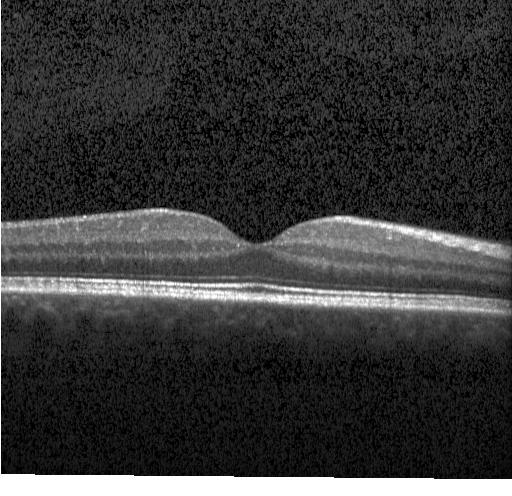

Heidelberg Spectralis · spectral-domain optical coherence tomography · fovea-centered · OCT line scan.
Finding: no evidence of choroidal neovascularization, diabetic macular edema, or drusen.